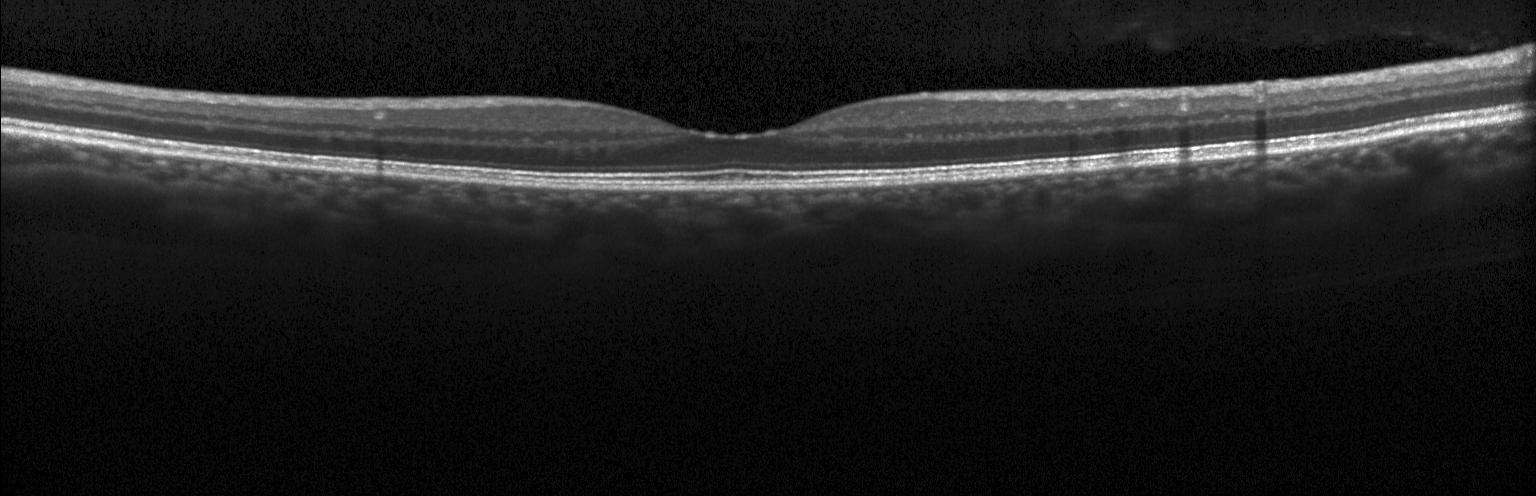
Retinal OCT B-scan; instrument: Heidelberg Spectralis — Diagnosis: neither choroidal neovascularization, diabetic macular edema, nor drusen.